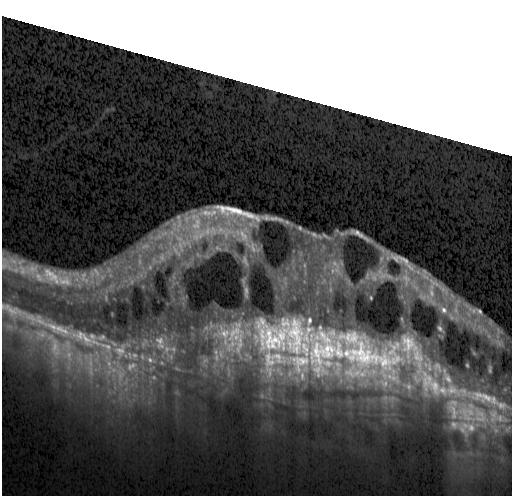
OCT B-scan · spectral-domain optical coherence tomography — Assessment: a choroidal neovascular membrane.